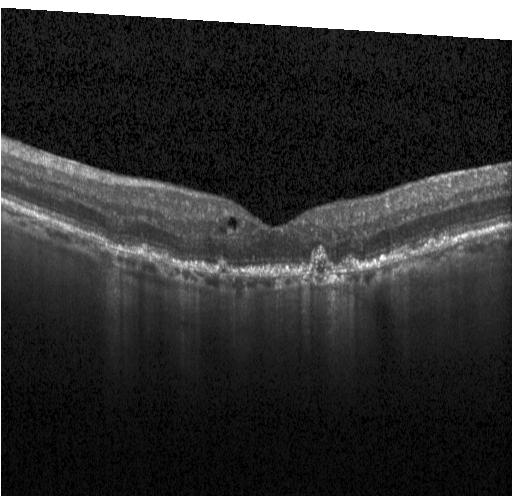

Spectral-domain optical coherence tomography, acquired on a Heidelberg Spectralis, retinal OCT cross-section — Diagnosis: choroidal neovascularization (CNV).